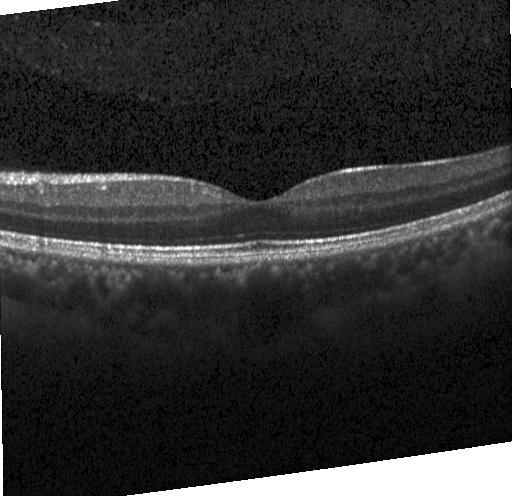 OCT B-scan
Finding: no CNV, no DME, and no drusen.